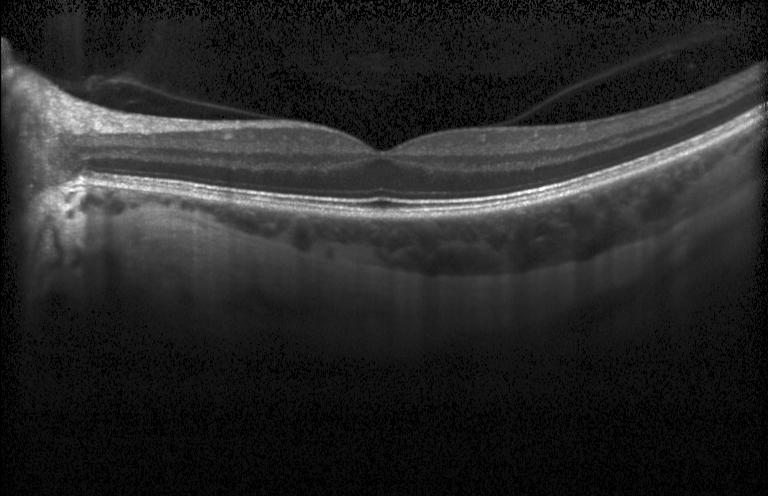 Retinal OCT B-scan. Through the macula. Spectral-domain optical coherence tomography
The scan shows no CNV, DME, or drusen.